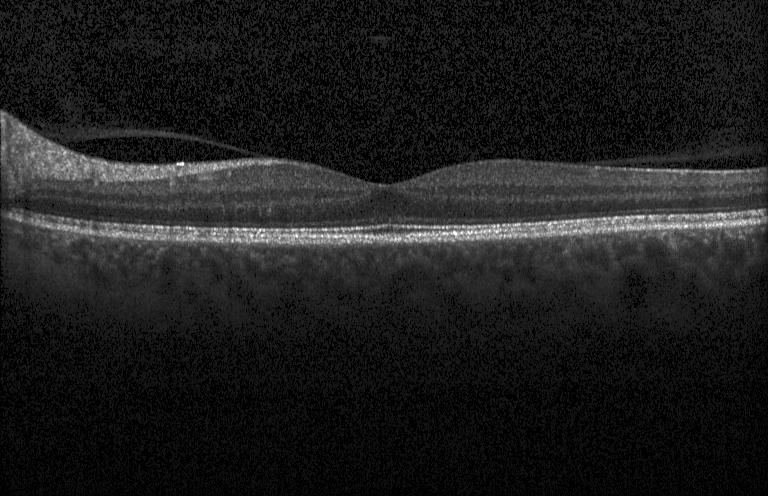

Instrument: Heidelberg Spectralis, spectral-domain optical coherence tomography, OCT line scan. Assessment: no choroidal neovascularization, diabetic macular edema, or drusen.